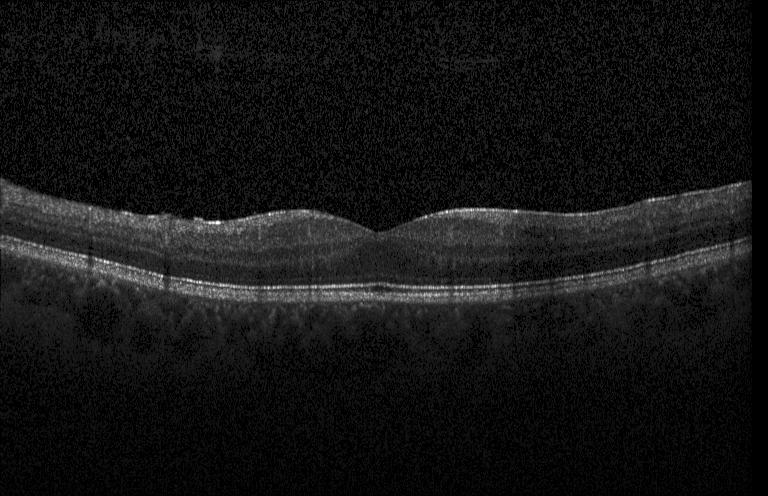

Retinal OCT cross-section. Instrument: Heidelberg Spectralis.
This B-scan demonstrates no choroidal neovascularization, no diabetic macular edema, and no drusen.